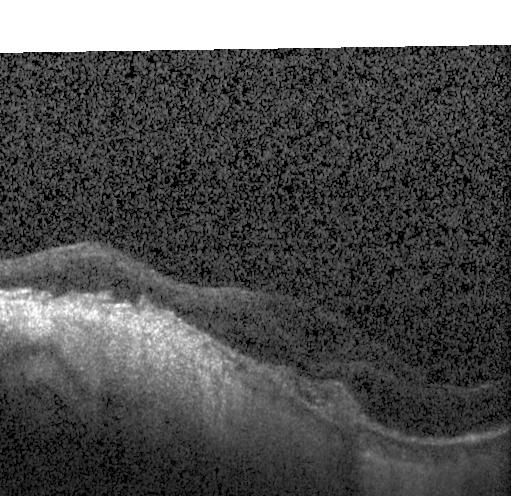 Spectral-domain OCT; Heidelberg Spectralis OCT system; OCT line scan.
Impression: a choroidal neovascular membrane.